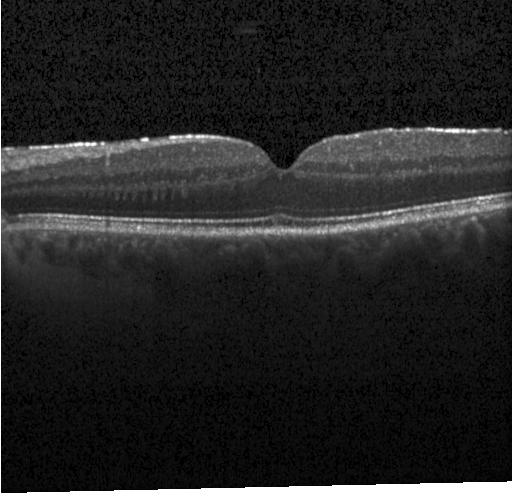

Finding: no evidence of CNV, DME, or drusen.